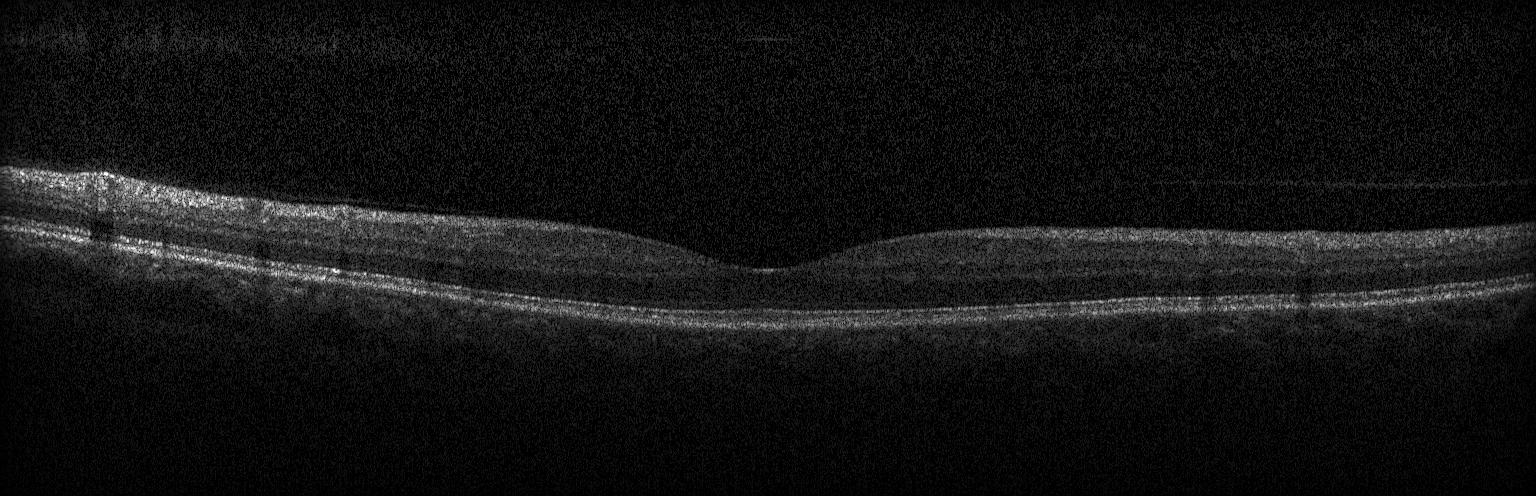 Acquired on a Heidelberg Spectralis; macular scan; spectral-domain OCT; optical coherence tomography B-scan.
Finding: neither choroidal neovascularization, diabetic macular edema, nor drusen.